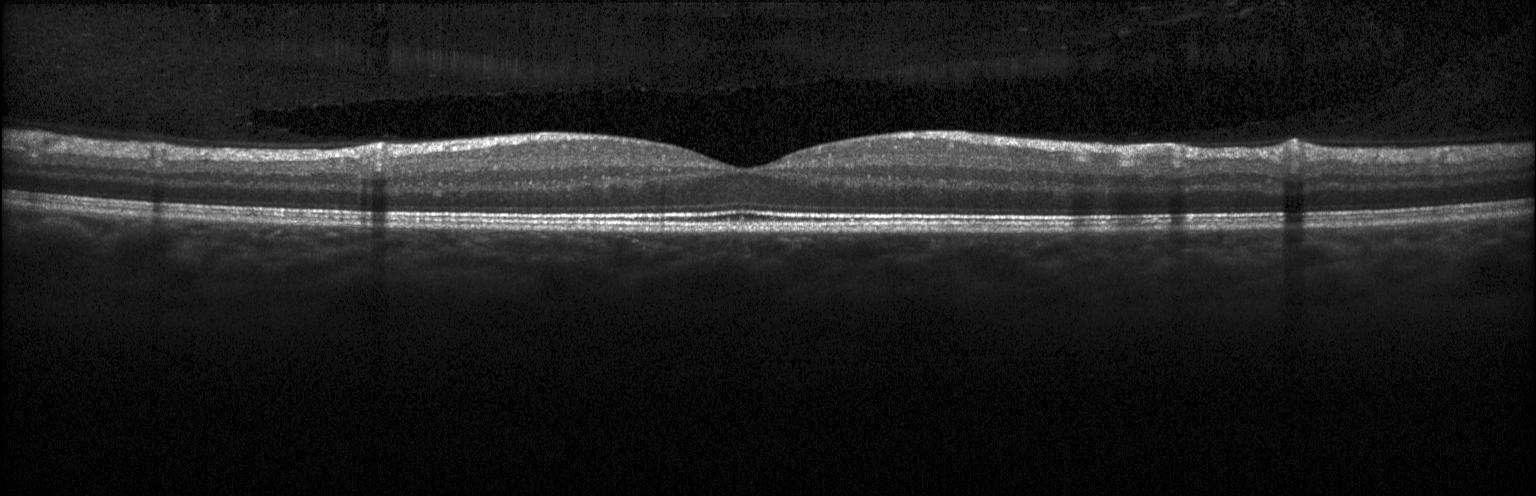

Spectral-domain optical coherence tomography; OCT line scan; centered on the fovea; Heidelberg Spectralis OCT system.
Diagnosis: neither choroidal neovascularization, diabetic macular edema, nor drusen.